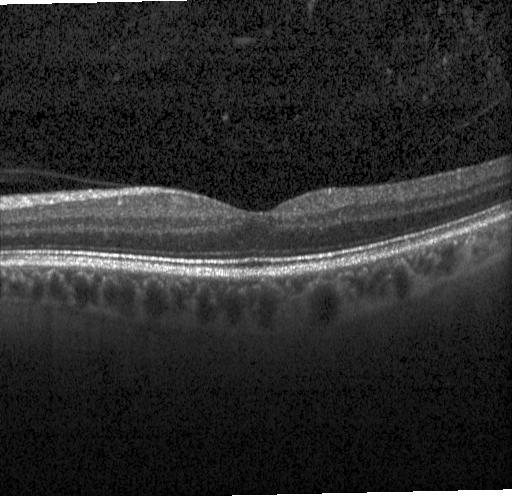
Spectral-domain optical coherence tomography. Optical coherence tomography B-scan. Macular scan — Diagnosis: no choroidal neovascularization, diabetic macular edema, or drusen.